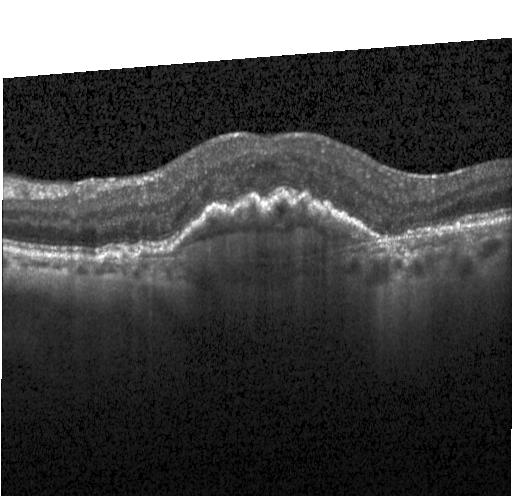 Spectral-domain optical coherence tomography, instrument: Heidelberg Spectralis, OCT B-scan, macular scan. Diagnosis: a choroidal neovascular membrane.